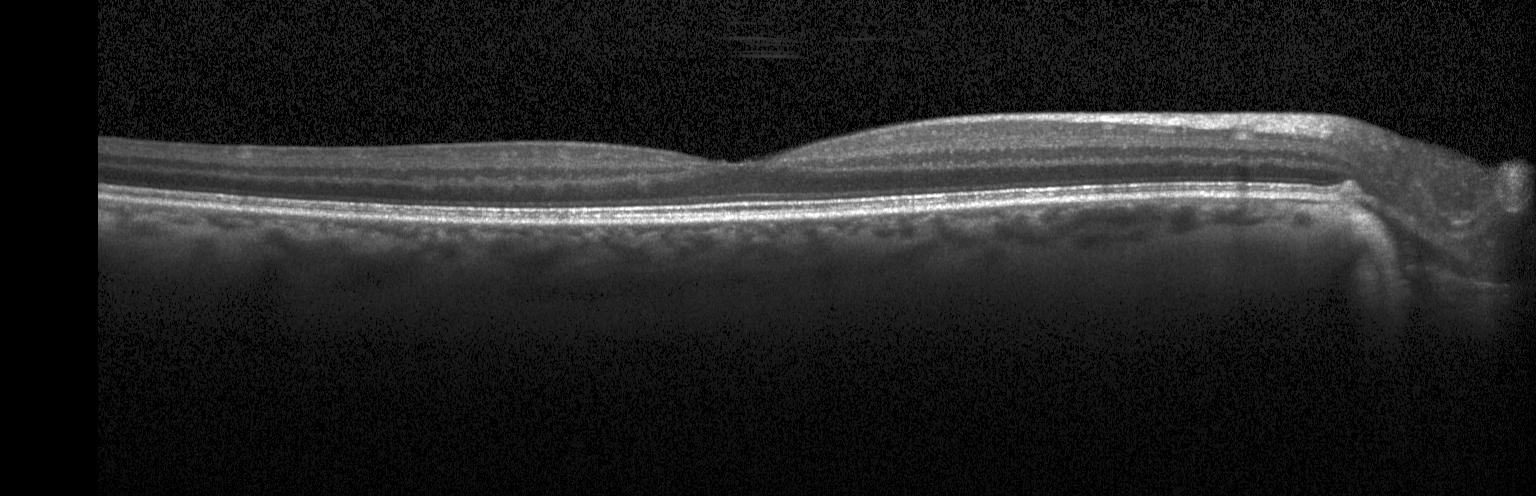

Heidelberg Spectralis; centered on the fovea; retinal OCT B-scan.
Assessment: no choroidal neovascularization, no diabetic macular edema, and no drusen.